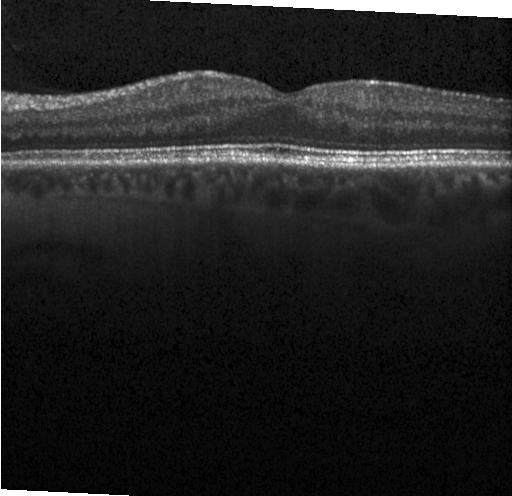 OCT finding: no CNV, no DME, and no drusen.